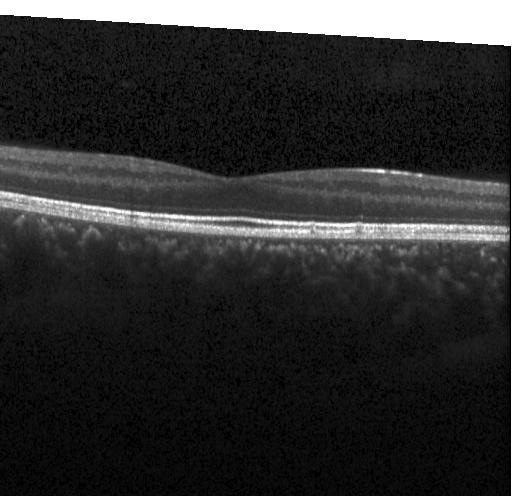 Retinal OCT cross-section · macular scan.
Impression: no evidence of choroidal neovascularization, diabetic macular edema, or drusen.